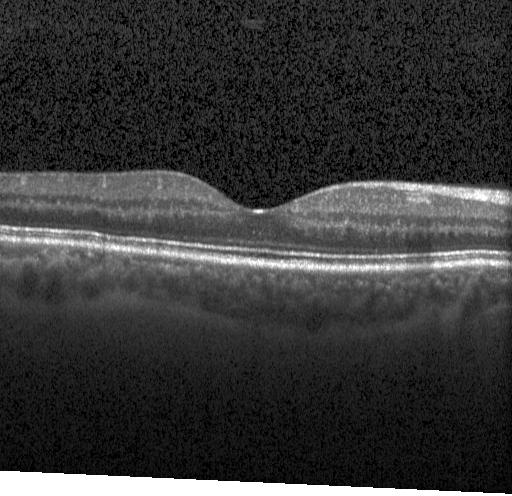 Acquired on a Heidelberg Spectralis; spectral-domain OCT; horizontal scan through the fovea; OCT line scan — Impression: no choroidal neovascularization, no diabetic macular edema, and no drusen.